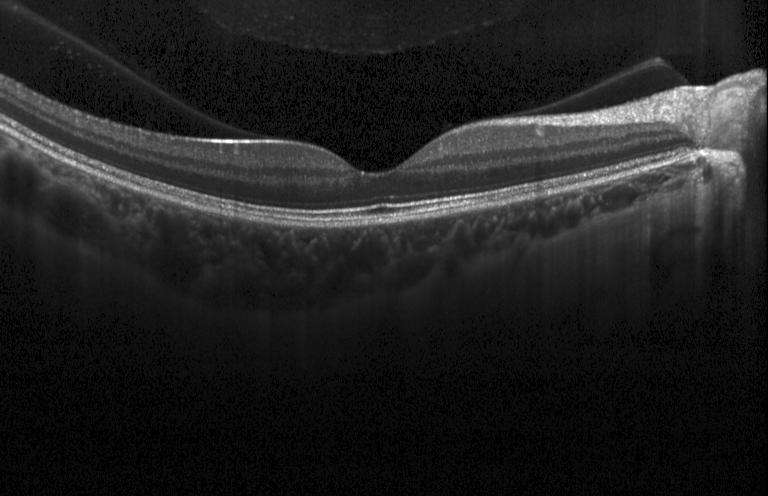
Retinal OCT cross-section; spectral-domain OCT.
Impression: no evidence of CNV, DME, or drusen.